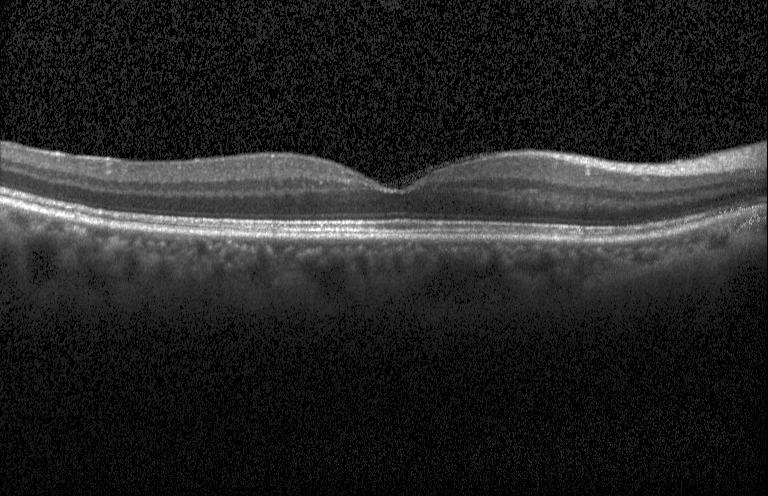 Spectral-domain optical coherence tomography, OCT B-scan, acquired on a Heidelberg Spectralis — OCT finding: no evidence of CNV, DME, or drusen.